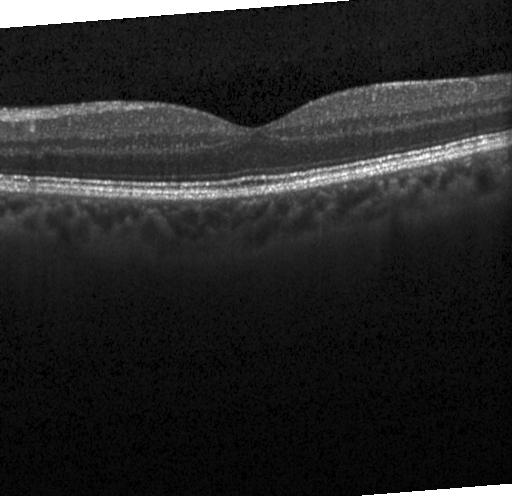
Optical coherence tomography scan
Macular OCT: no choroidal neovascularization, no diabetic macular edema, and no drusen.